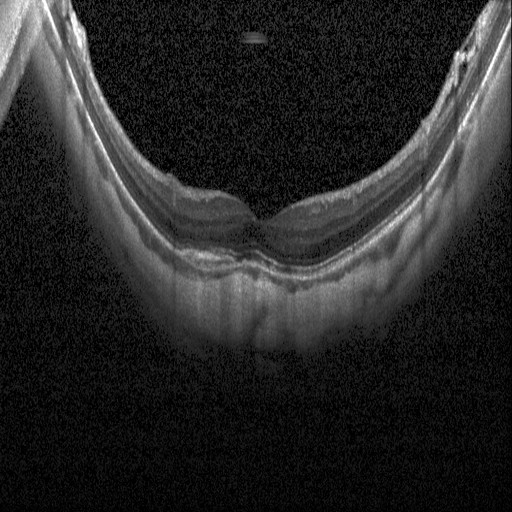 Spectral-domain optical coherence tomography; OCT B-scan
Impression: DME.